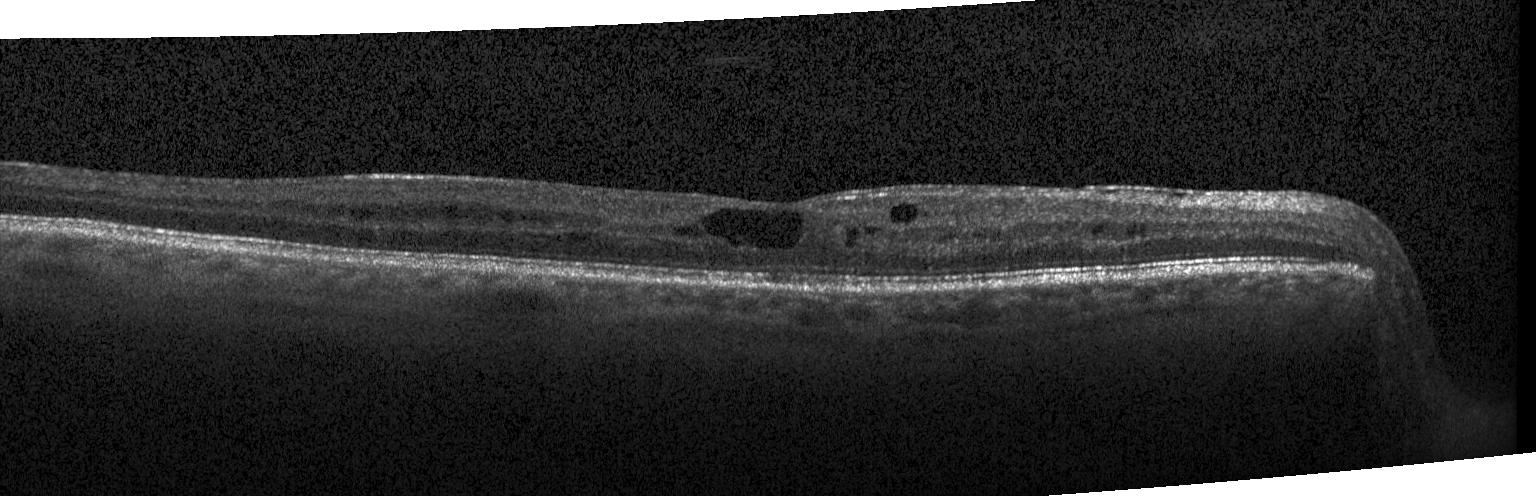

Diagnosis: DME.